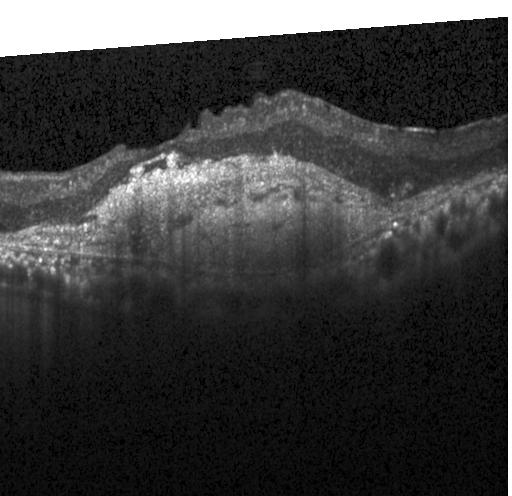 Heidelberg Spectralis. Optical coherence tomography B-scan — Macular OCT: a choroidal neovascular membrane.